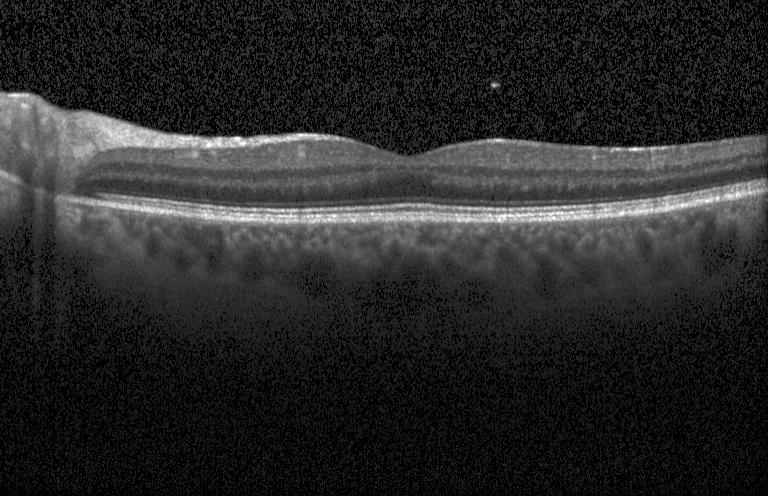

Centered on the fovea, SD-OCT, retinal OCT cross-section.
Dx: neither CNV, DME, nor drusen.